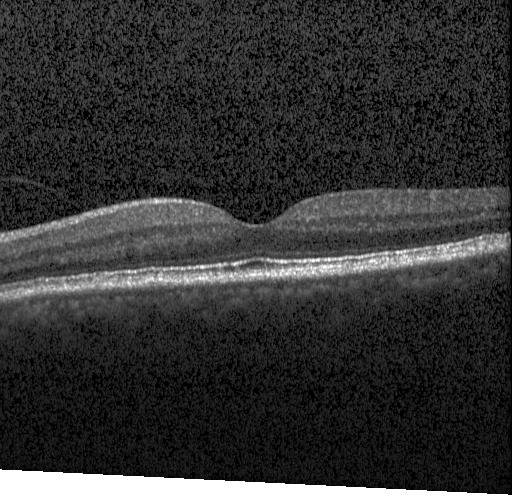

OCT line scan; spectral-domain OCT.
Assessment: neither choroidal neovascularization, diabetic macular edema, nor drusen.